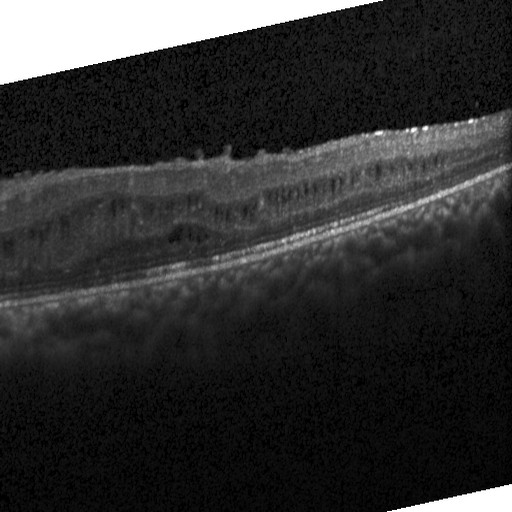 Retinal OCT cross-section — Impression: diabetic macular edema.